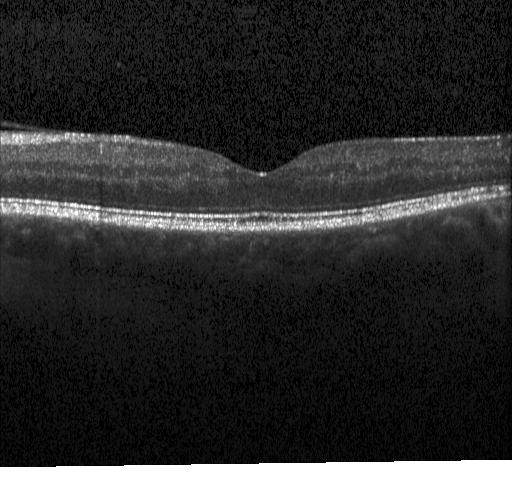 Macular scan · Heidelberg Spectralis · optical coherence tomography B-scan. Finding: neither choroidal neovascularization, diabetic macular edema, nor drusen.